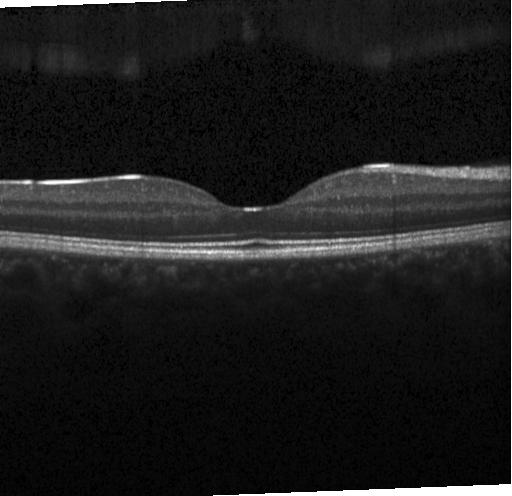
OCT line scan. Horizontal scan through the fovea. Spectral-domain optical coherence tomography — No choroidal neovascularization, no diabetic macular edema, and no drusen.